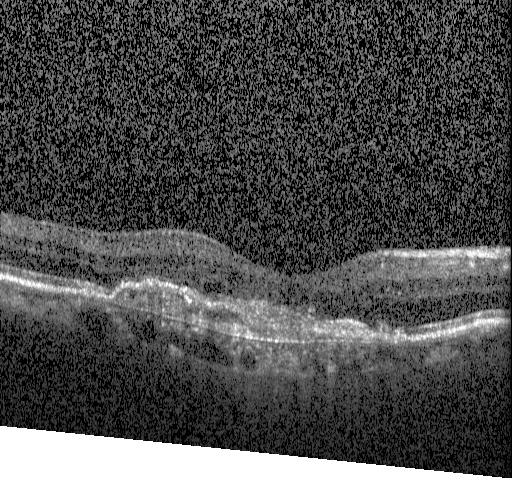 OCT B-scan. Instrument: Heidelberg Spectralis. Through the macula — Diagnosis: a choroidal neovascular membrane.